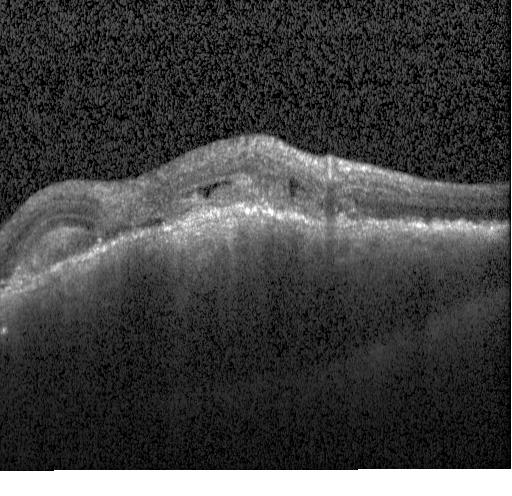 Impression: CNV.